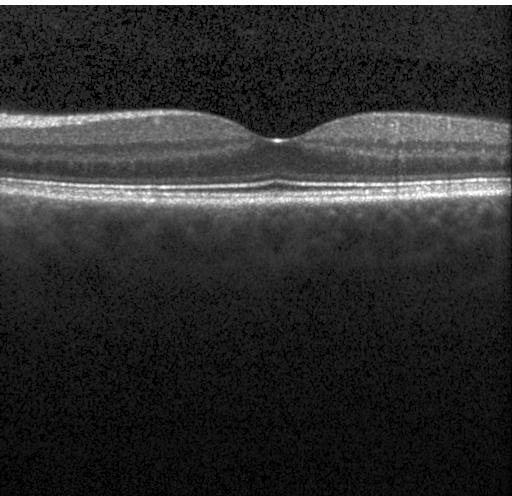
Heidelberg Spectralis OCT system; OCT line scan; macular scan
Finding: no CNV, no DME, and no drusen.